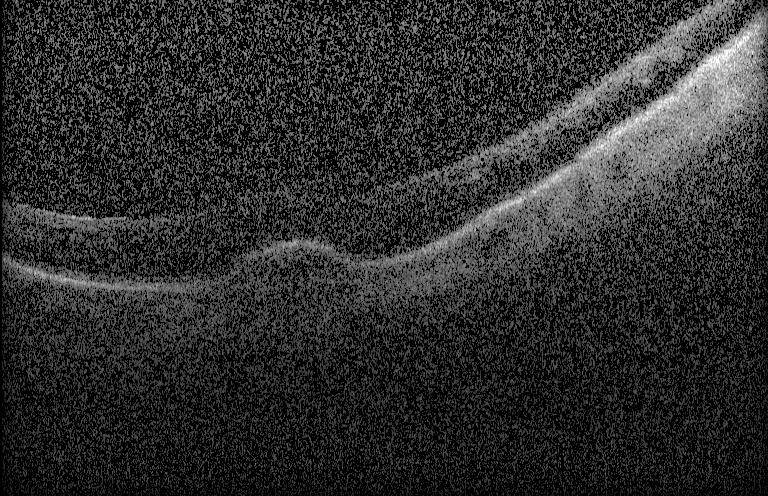
Optical coherence tomography scan · spectral-domain optical coherence tomography · through the macula · Heidelberg Spectralis — Finding: CNV.